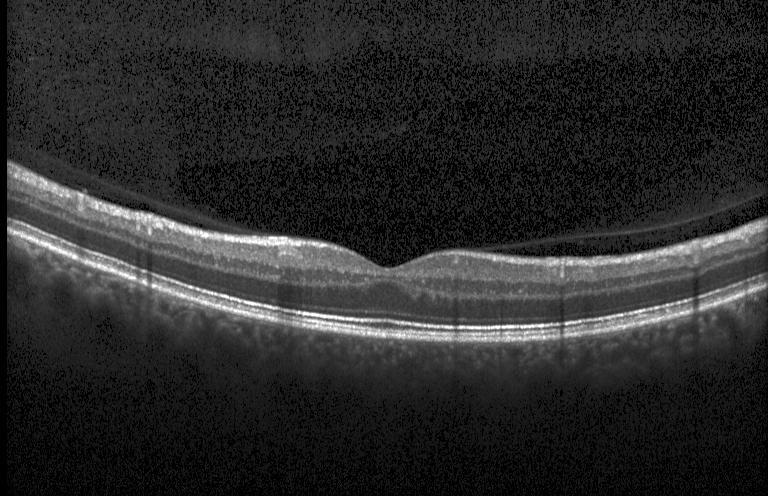 OCT finding: no choroidal neovascularization, no diabetic macular edema, and no drusen.